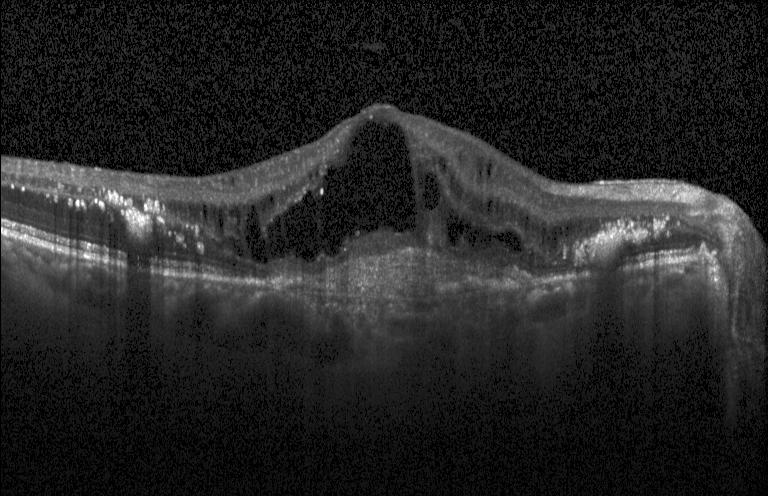

Diagnosis: choroidal neovascularization (CNV).